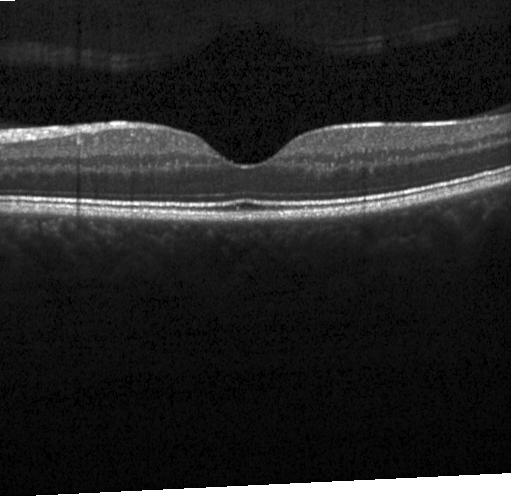 Optical coherence tomography scan. Horizontal scan through the fovea. Acquired on a Heidelberg Spectralis.
OCT finding: neither CNV, DME, nor drusen.